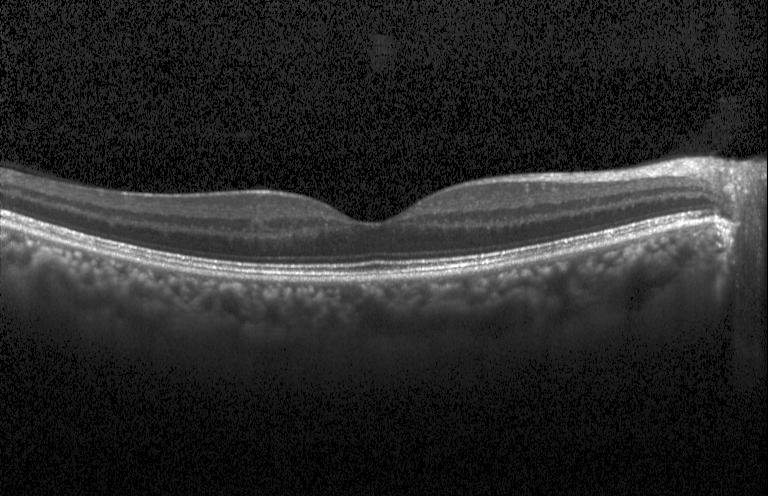

Spectral-domain OCT. Retinal OCT cross-section
Impression: no evidence of choroidal neovascularization, diabetic macular edema, or drusen.